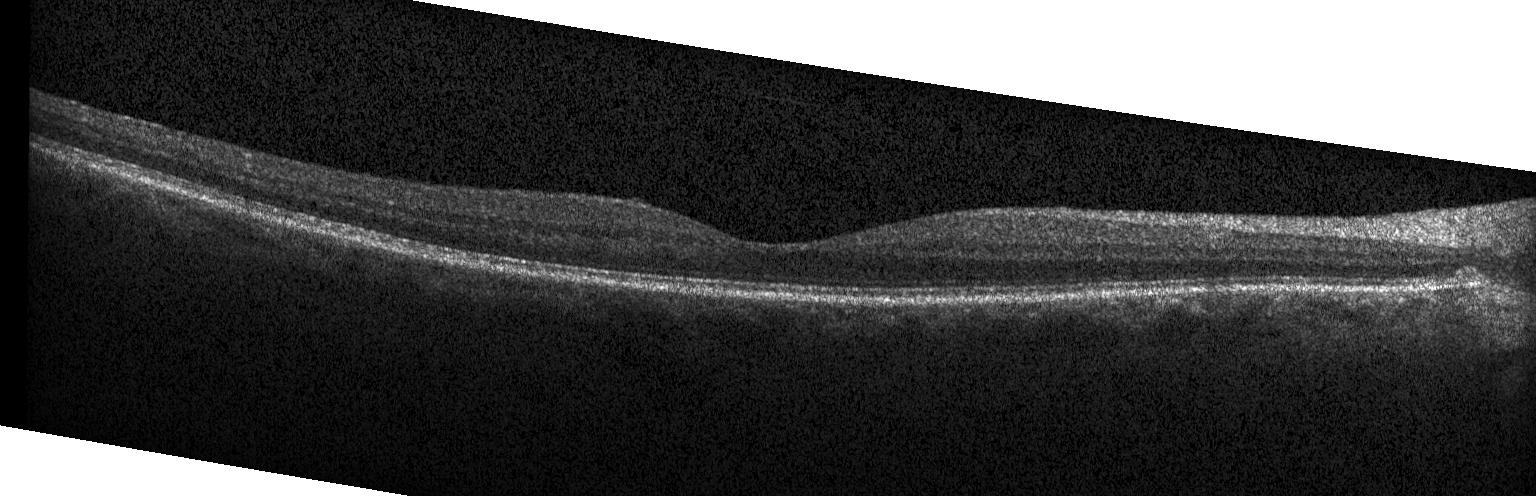 OCT scan showing no evidence of choroidal neovascularization, diabetic macular edema, or drusen.